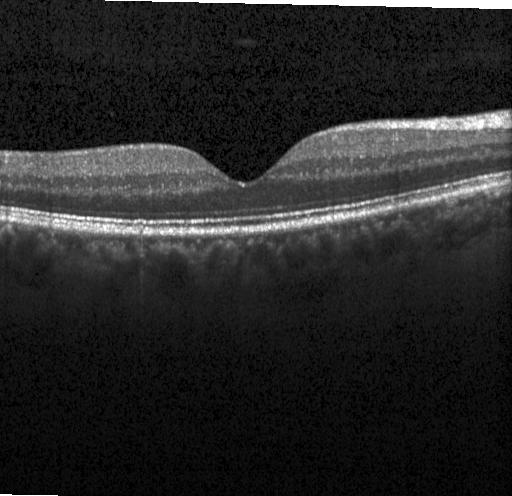 Optical coherence tomography scan, acquired on a Heidelberg Spectralis, horizontal scan through the fovea — This B-scan demonstrates no CNV, DME, or drusen.